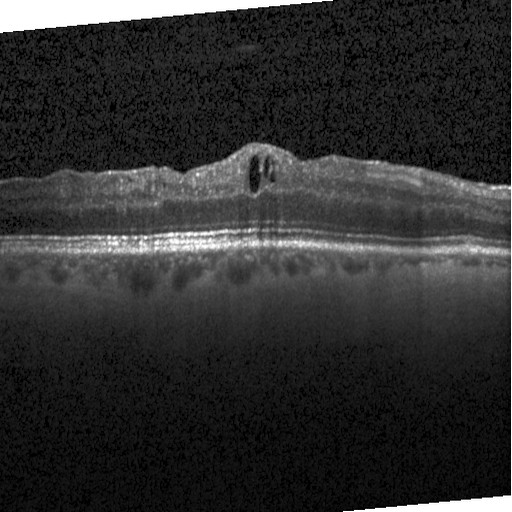 Optical coherence tomography B-scan, acquired on a Heidelberg Spectralis, macular scan
Finding: diabetic macular edema.